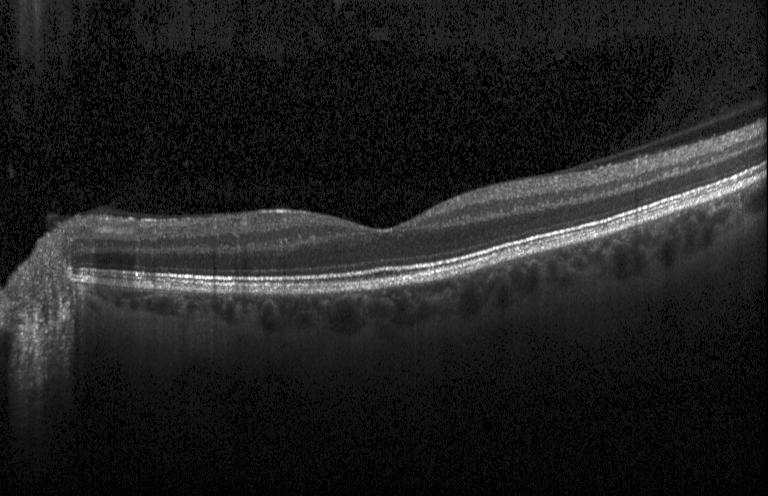

Optical coherence tomography B-scan. SD-OCT. Through the macula. Acquired on a Heidelberg Spectralis — Assessment: neither choroidal neovascularization, diabetic macular edema, nor drusen.